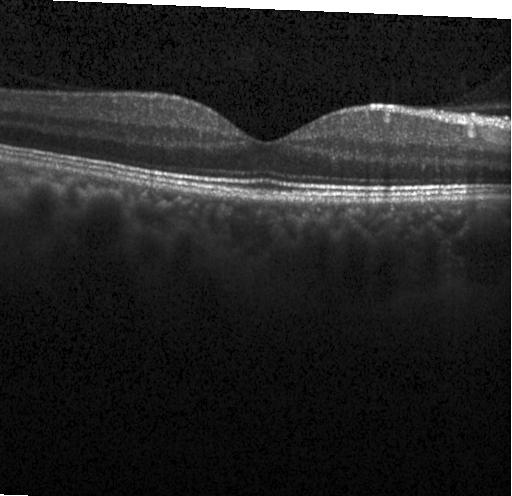
SD-OCT; OCT line scan; Heidelberg Spectralis.
This B-scan demonstrates no choroidal neovascularization, no diabetic macular edema, and no drusen.